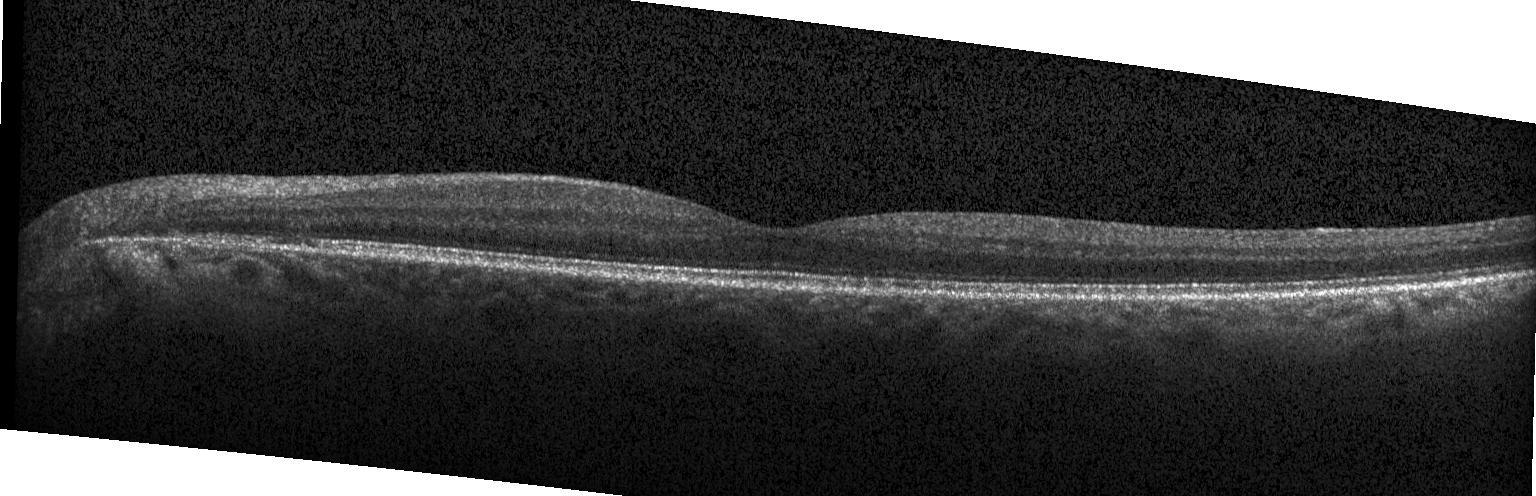
Heidelberg Spectralis; spectral-domain optical coherence tomography; OCT B-scan; through the macula.
Diagnosis: no choroidal neovascularization, diabetic macular edema, or drusen.